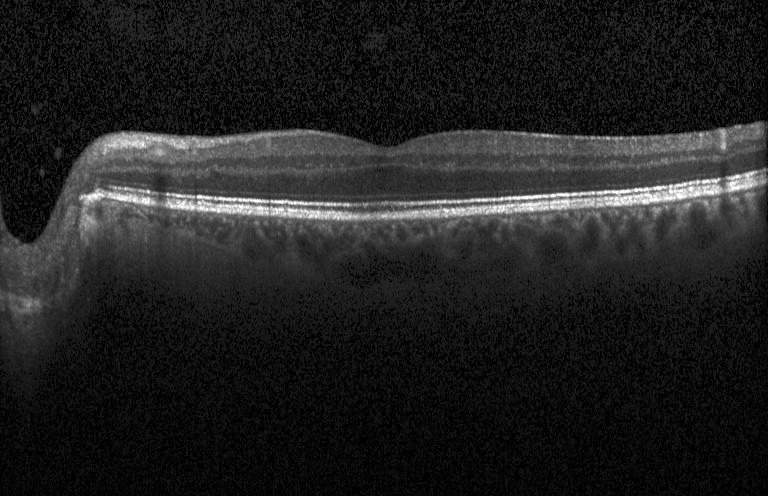
Optical coherence tomography B-scan · SD-OCT · Heidelberg Spectralis OCT system.
Finding: no CNV, DME, or drusen.